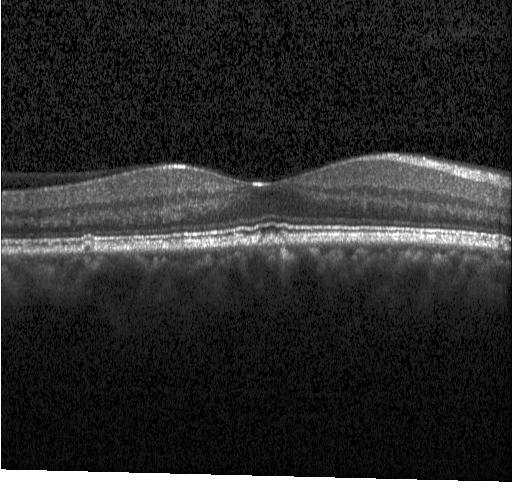

Spectral-domain OCT · optical coherence tomography B-scan
Diagnosis: multiple drusen.